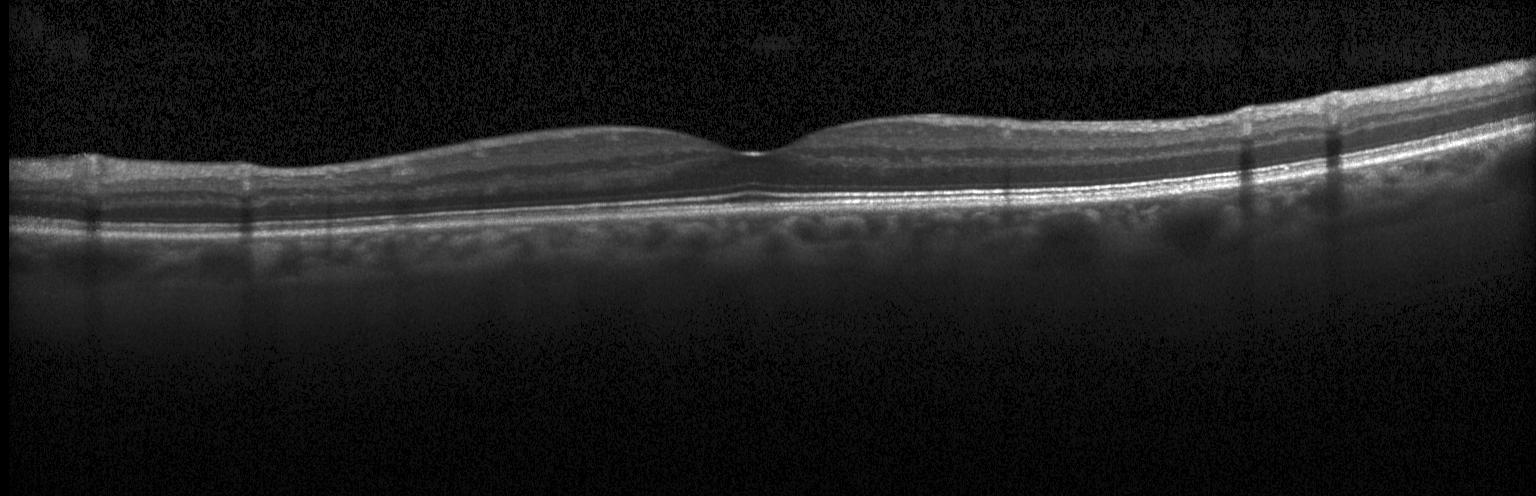

Optical coherence tomography B-scan, SD-OCT, centered on the fovea. Impression: no choroidal neovascularization, diabetic macular edema, or drusen.